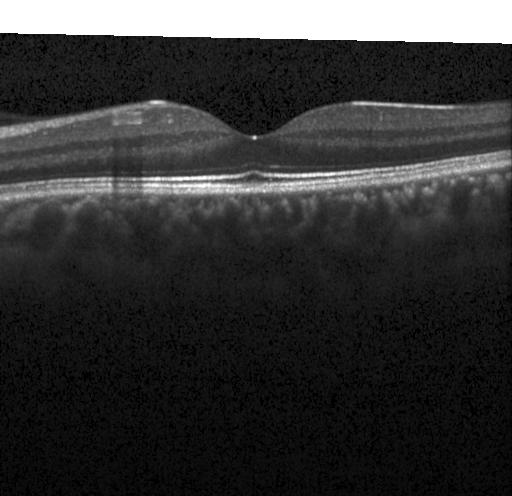 Macular OCT: neither choroidal neovascularization, diabetic macular edema, nor drusen.